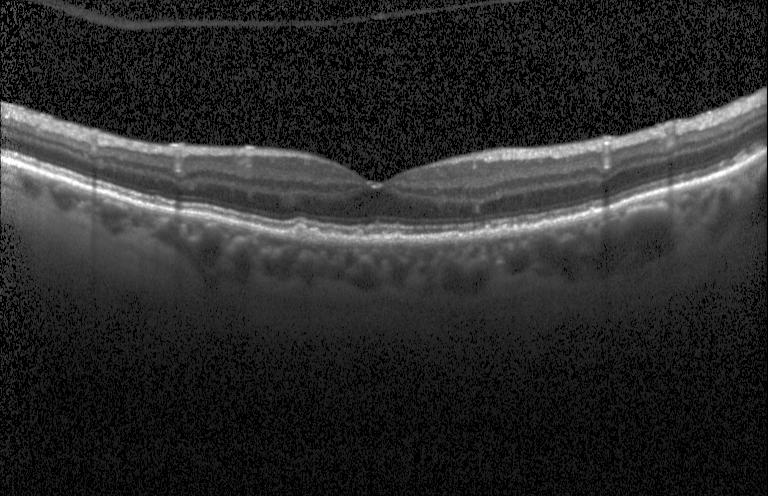 Heidelberg Spectralis OCT system · through the macula · retinal OCT cross-section · SD-OCT. Dx: sub-RPE drusenoid deposits.